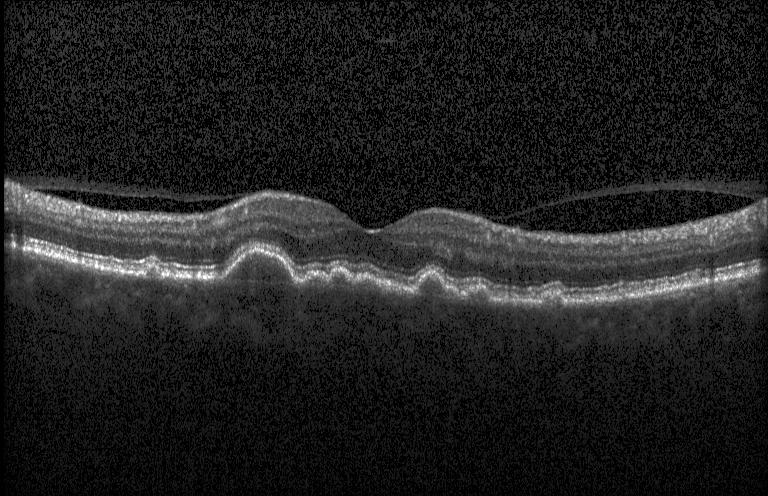
OCT line scan — This B-scan demonstrates multiple drusen.